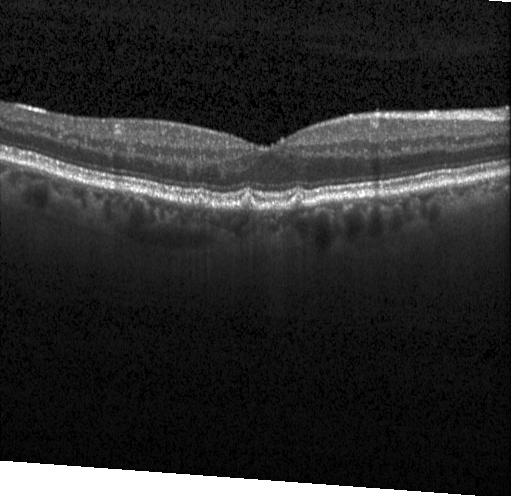
Finding: multiple drusen.